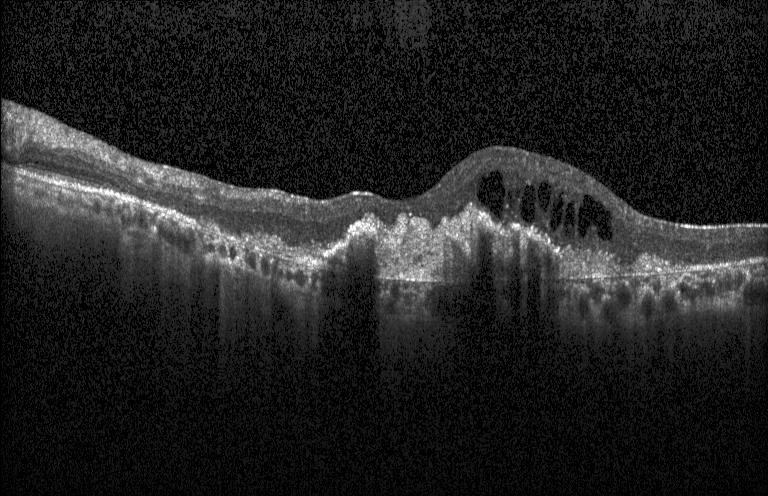

Acquired on a Heidelberg Spectralis · optical coherence tomography B-scan · spectral-domain optical coherence tomography
Macular OCT: a choroidal neovascular membrane.